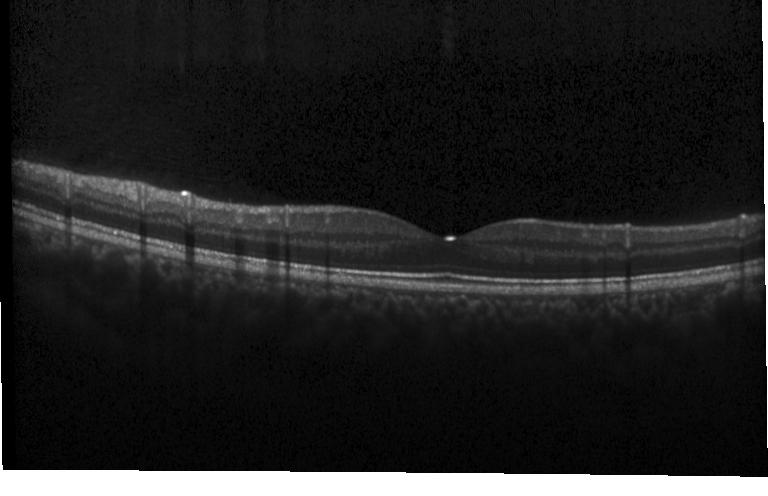
Optical coherence tomography scan — Diagnosis: no choroidal neovascularization, no diabetic macular edema, and no drusen.